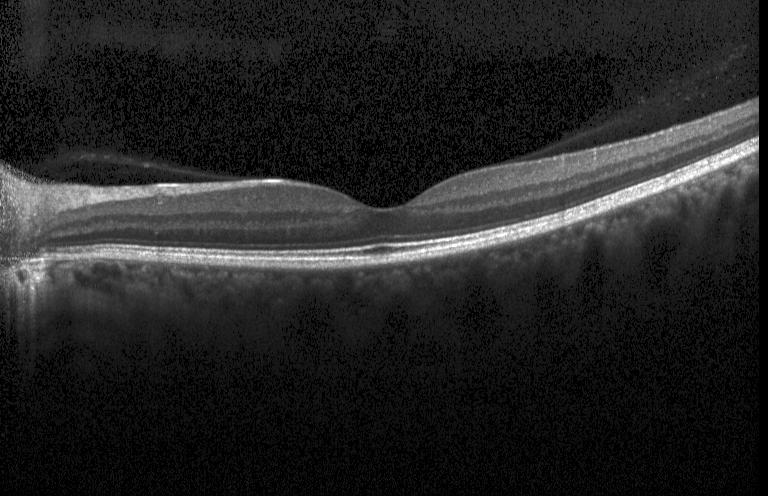
Macular scan. Retinal OCT B-scan. Heidelberg Spectralis OCT system — Finding: no evidence of choroidal neovascularization, diabetic macular edema, or drusen.